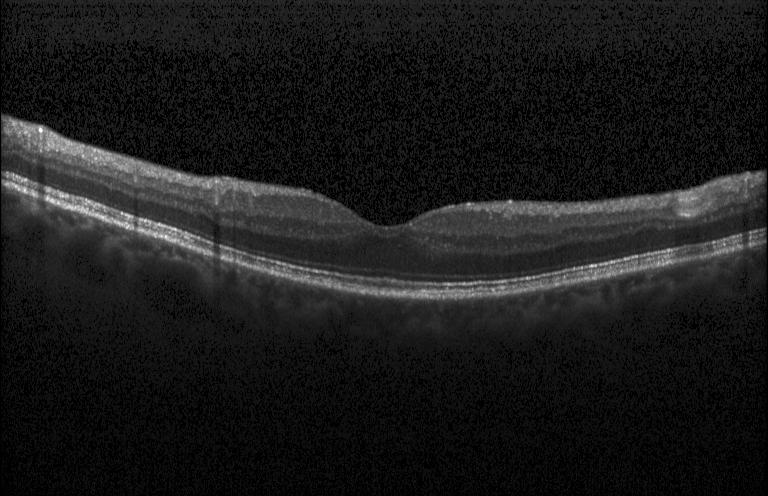

Impression: no choroidal neovascularization, diabetic macular edema, or drusen.